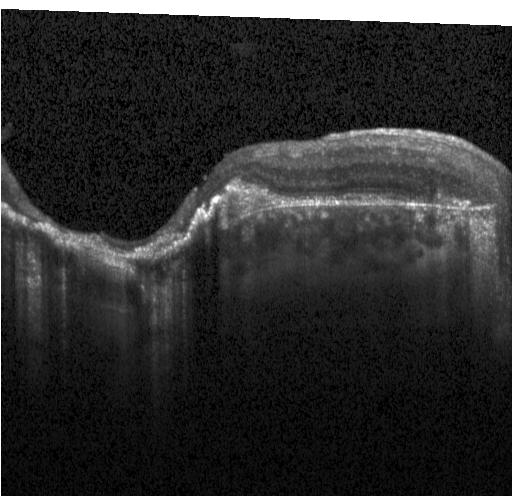

Heidelberg Spectralis · retinal OCT cross-section — Assessment: a choroidal neovascular membrane.